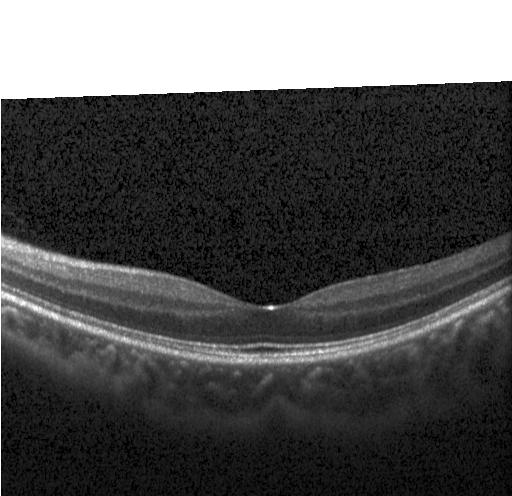
Dx: no choroidal neovascularization, diabetic macular edema, or drusen.